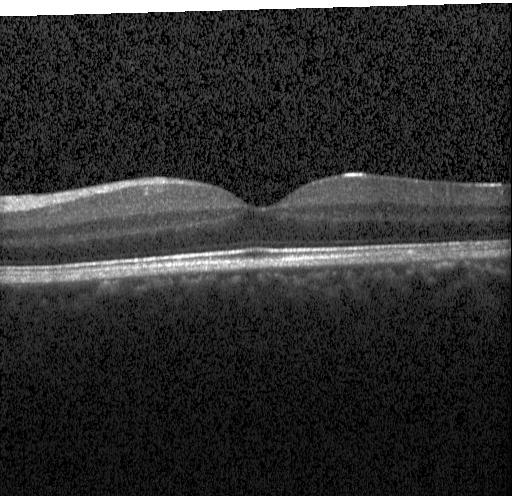
The scan shows no choroidal neovascularization, no diabetic macular edema, and no drusen.